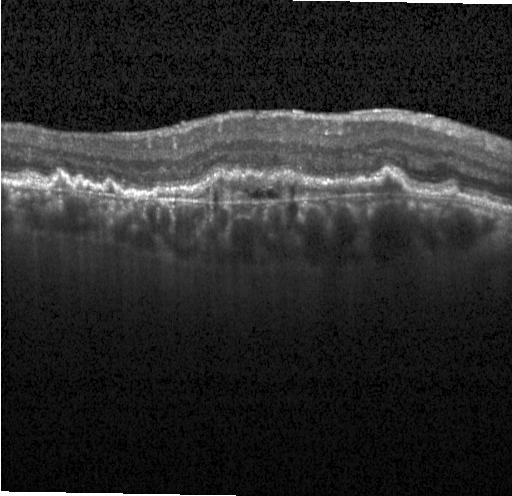 Retinal OCT cross-section
Impression: CNV.